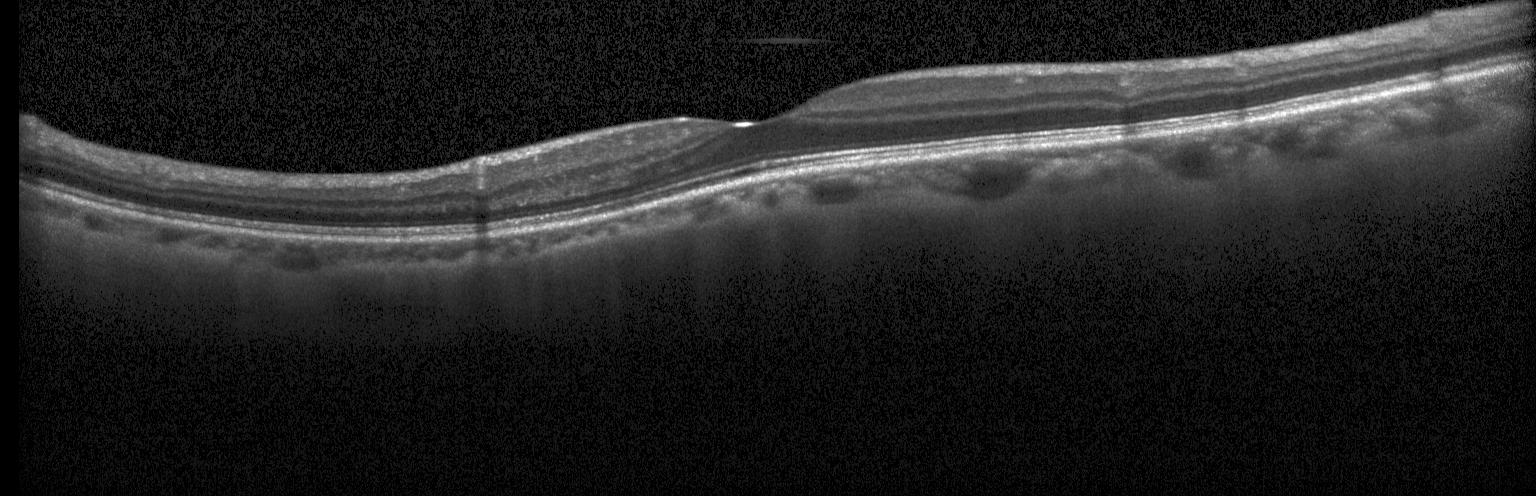
Retinal OCT cross-section showing neither choroidal neovascularization, diabetic macular edema, nor drusen.